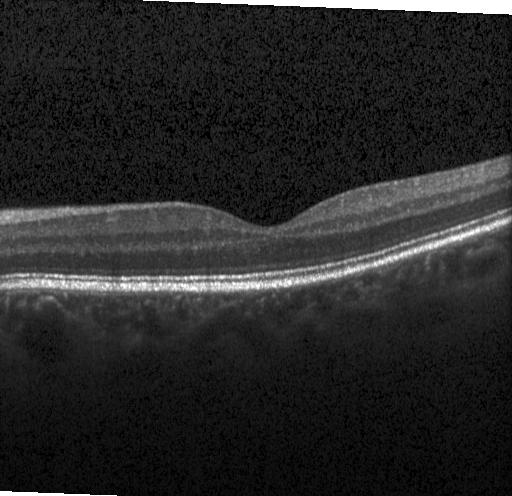
OCT scan showing no choroidal neovascularization, diabetic macular edema, or drusen.